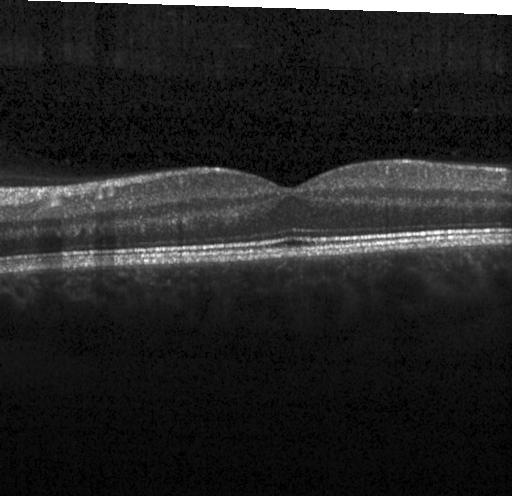 Impression: no CNV, DME, or drusen.